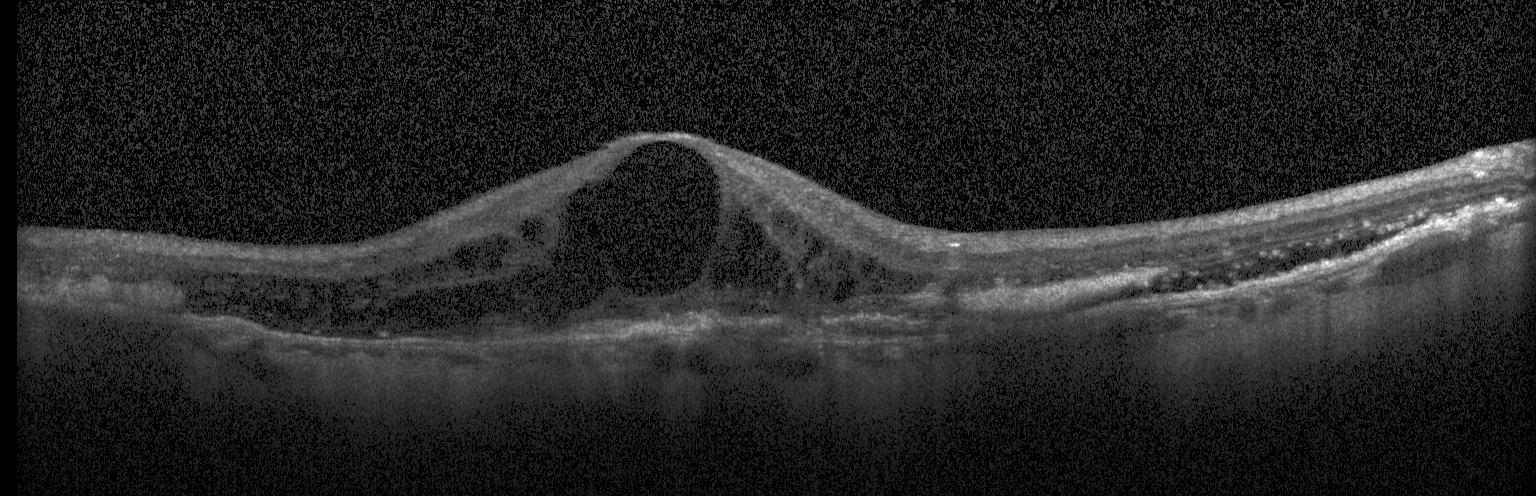

OCT line scan
Assessment: a choroidal neovascular membrane.